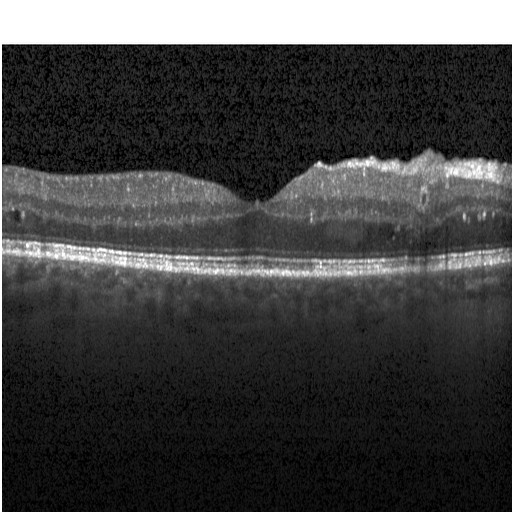

Instrument: Heidelberg Spectralis, retinal OCT cross-section. This B-scan demonstrates diabetic macular edema.